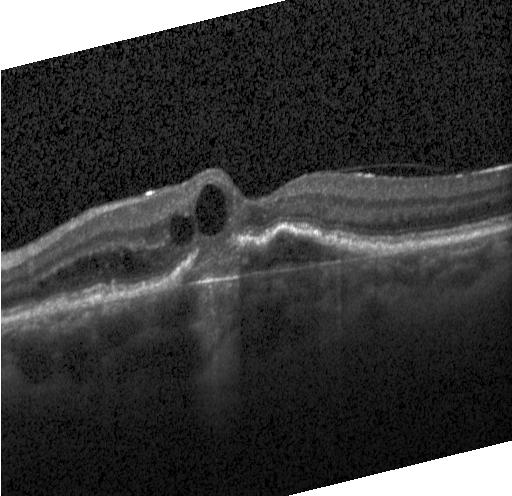

Retinal OCT cross-section
Assessment: choroidal neovascularization.